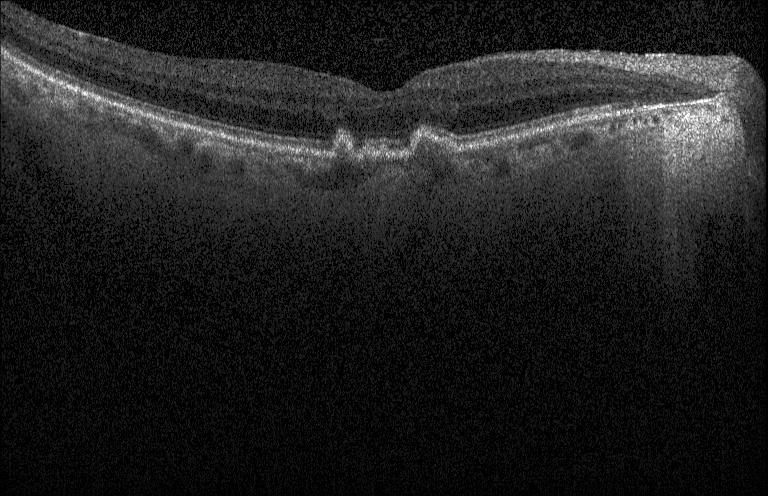 OCT B-scan. Impression: sub-RPE drusenoid deposits.